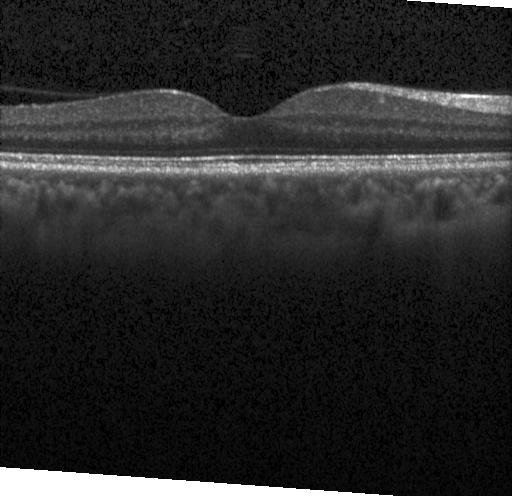
Assessment: no choroidal neovascularization, diabetic macular edema, or drusen.